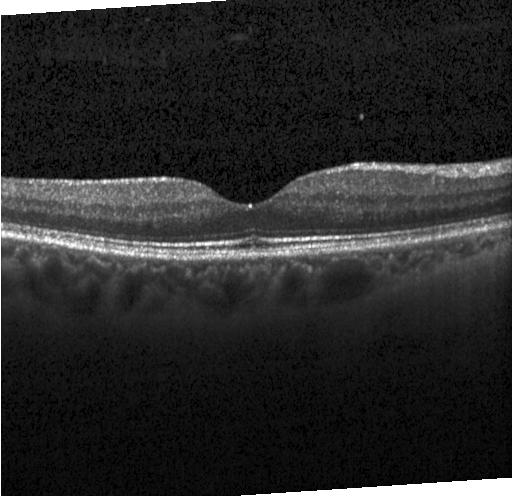
SD-OCT · Heidelberg Spectralis · retinal OCT cross-section — This B-scan demonstrates no choroidal neovascularization, no diabetic macular edema, and no drusen.